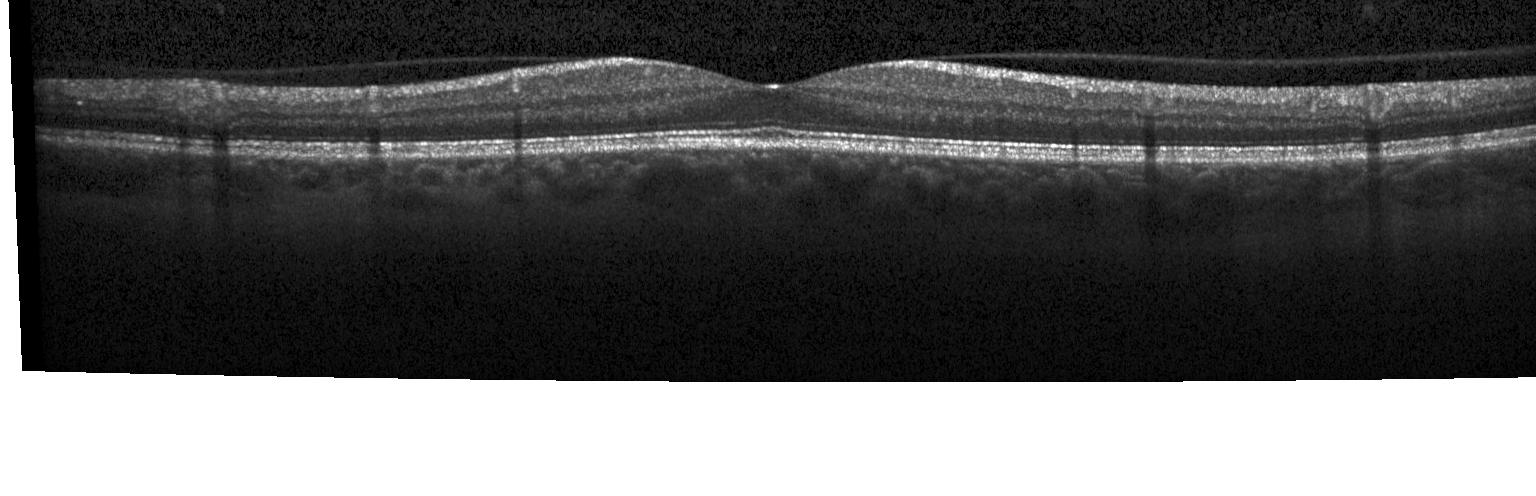
Retinal OCT cross-section showing neither choroidal neovascularization, diabetic macular edema, nor drusen.